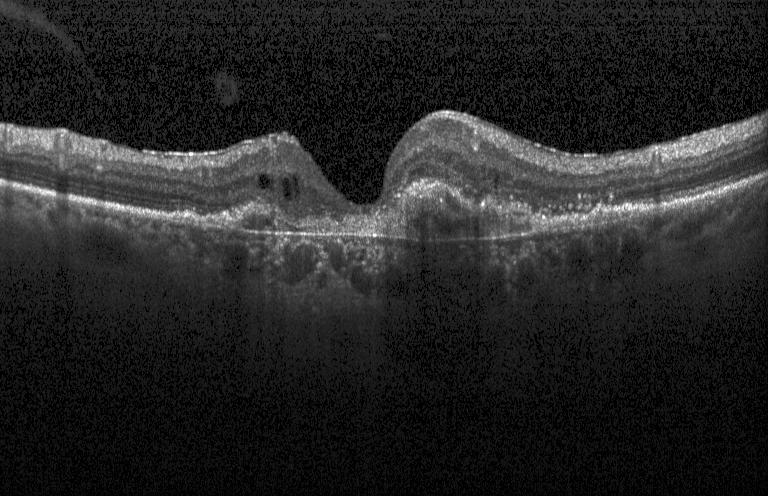 Spectral-domain optical coherence tomography, OCT line scan, fovea-centered, acquired on a Heidelberg Spectralis. Diagnosis: choroidal neovascularization.